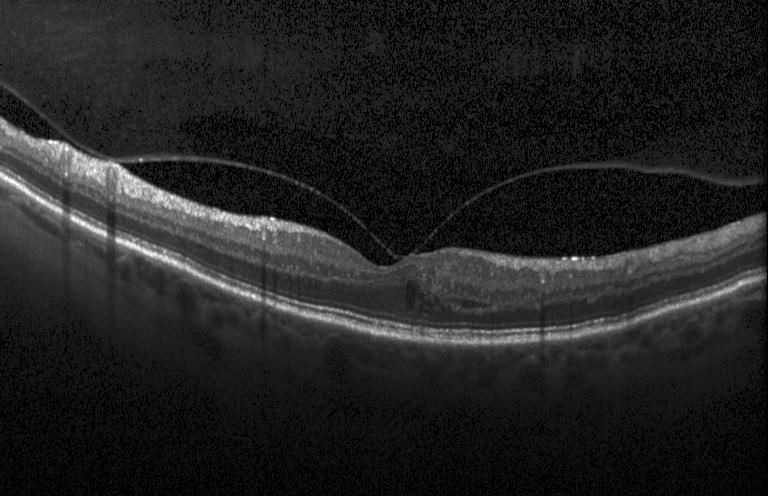

Centered on the fovea; acquired on a Heidelberg Spectralis; retinal OCT B-scan. OCT finding: diabetic macular edema (DME).